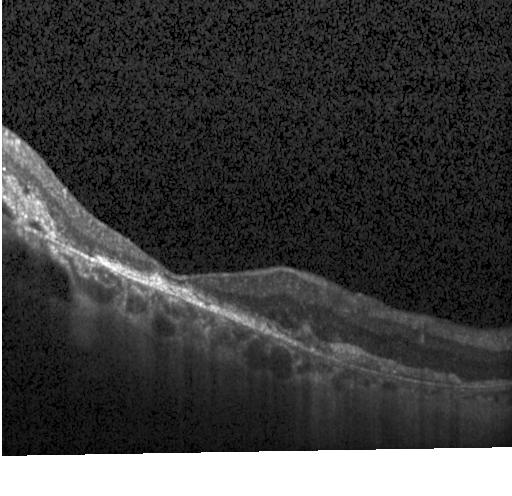

The scan shows choroidal neovascularization (CNV).